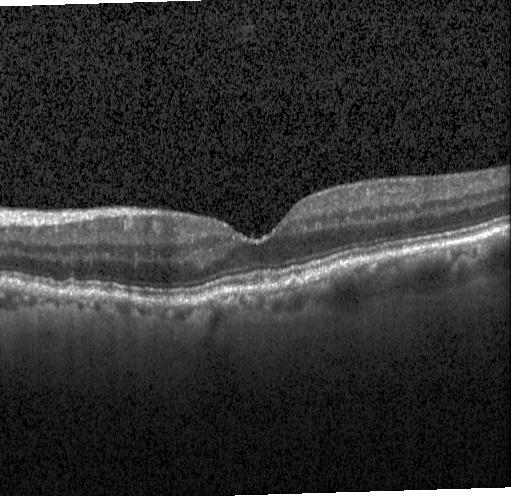

OCT finding: sub-RPE drusenoid deposits.